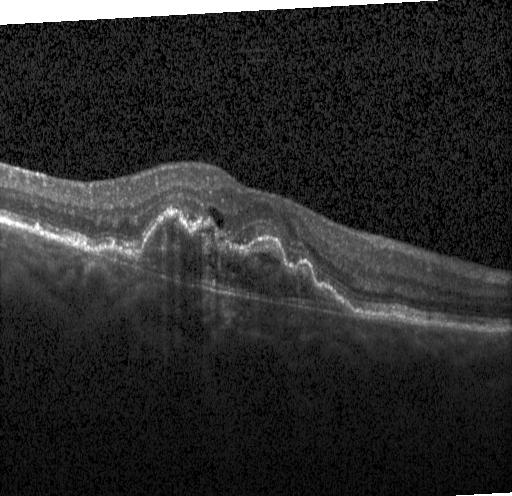
OCT scan showing choroidal neovascularization (CNV).